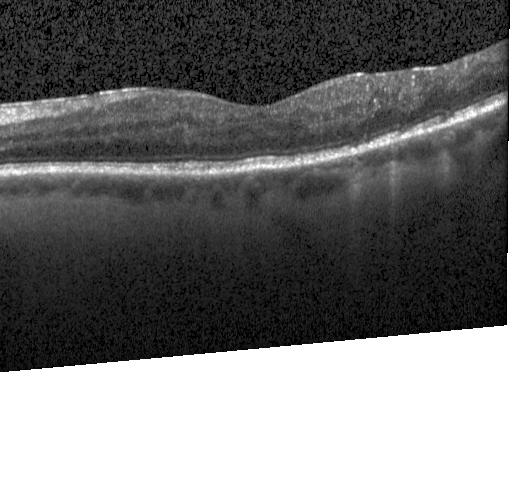
Heidelberg Spectralis OCT system. Optical coherence tomography B-scan. Fovea-centered — Diabetic macular edema.